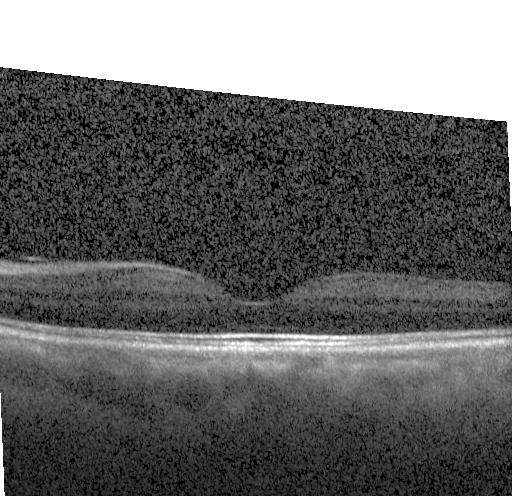 Macular OCT: no choroidal neovascularization, no diabetic macular edema, and no drusen.